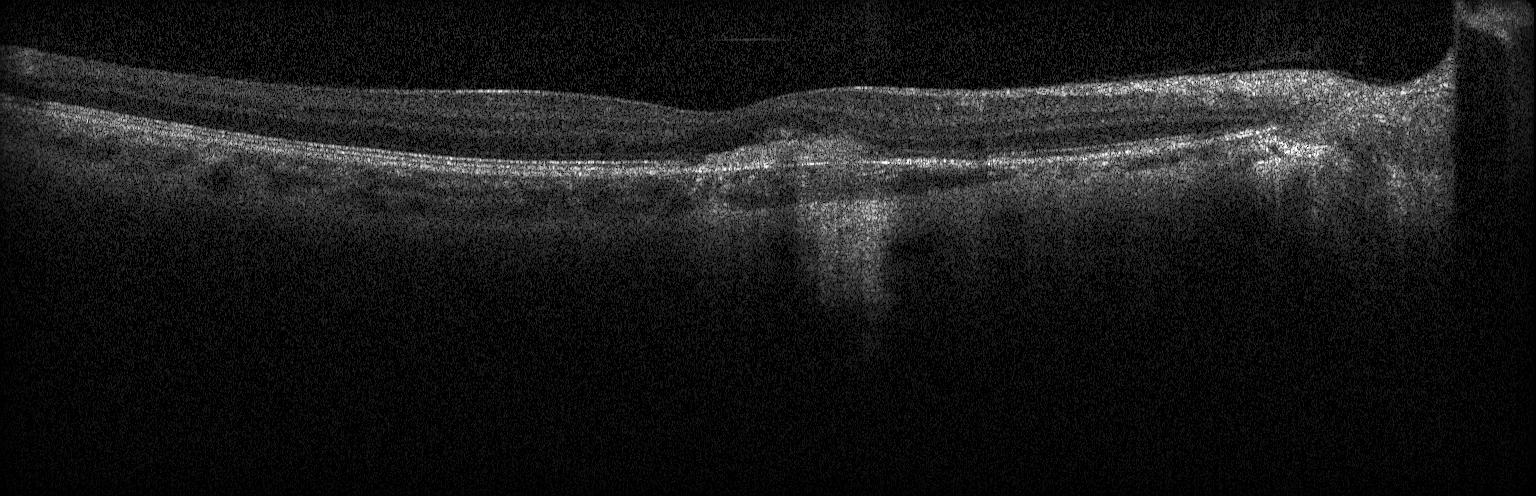
Fovea-centered; spectral-domain optical coherence tomography; Heidelberg Spectralis; optical coherence tomography scan.
Assessment: a choroidal neovascular membrane.